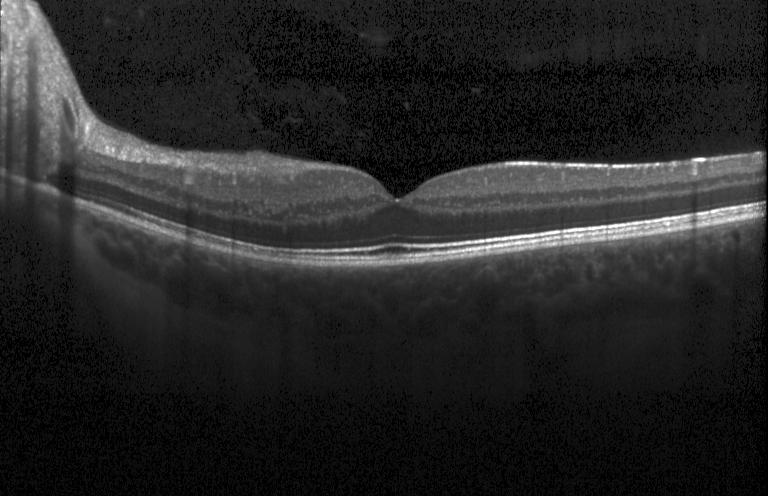 Spectral-domain OCT; optical coherence tomography B-scan
This B-scan demonstrates no evidence of choroidal neovascularization, diabetic macular edema, or drusen.